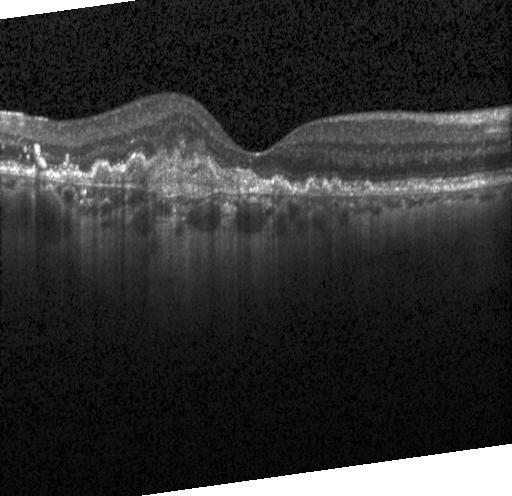 Macular scan · OCT B-scan.
Dx: a choroidal neovascular membrane.